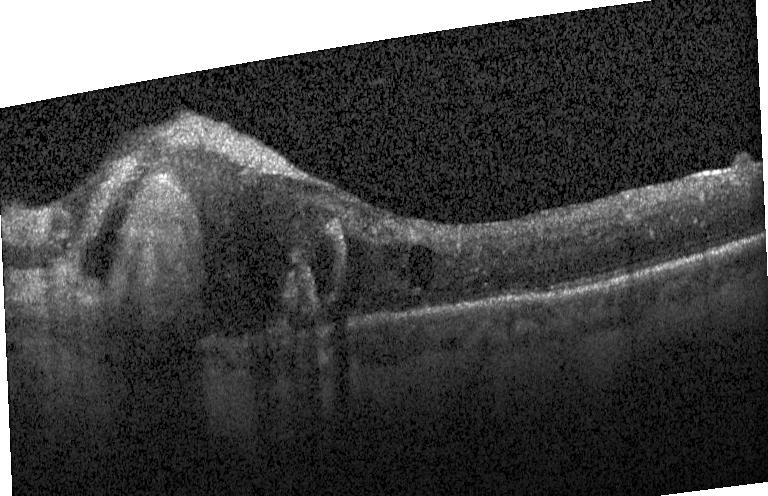
Optical coherence tomography B-scan — Macular OCT: choroidal neovascularization (CNV).